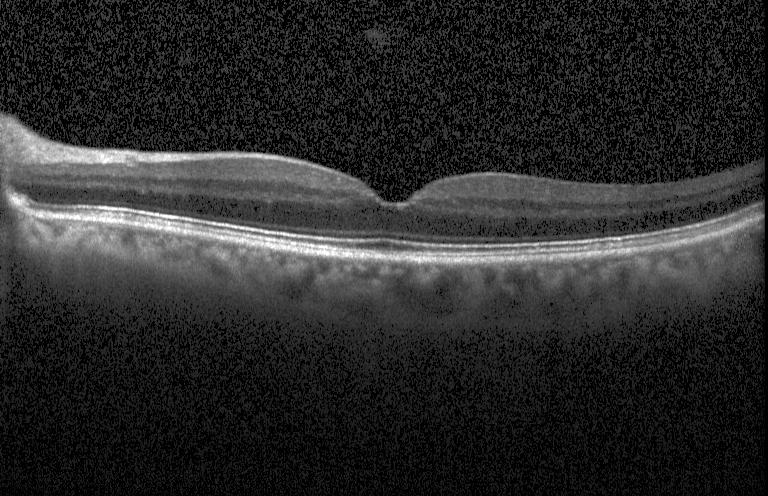 Retinal OCT cross-section, centered on the fovea, Heidelberg Spectralis.
Diagnosis: neither CNV, DME, nor drusen.